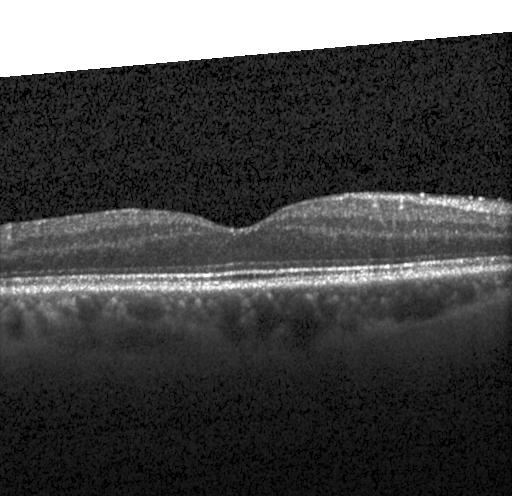

Optical coherence tomography scan
Dx: no choroidal neovascularization, diabetic macular edema, or drusen.